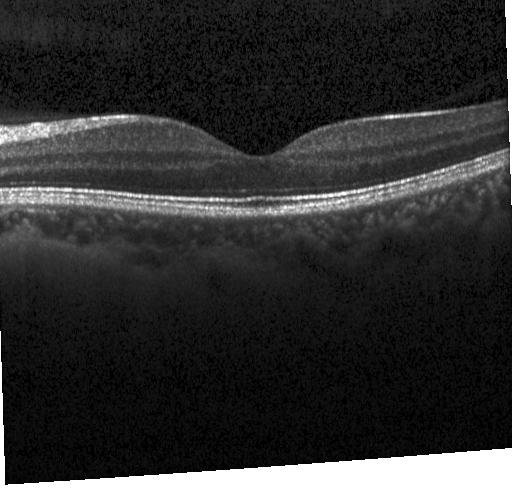

OCT B-scan showing no CNV, DME, or drusen.